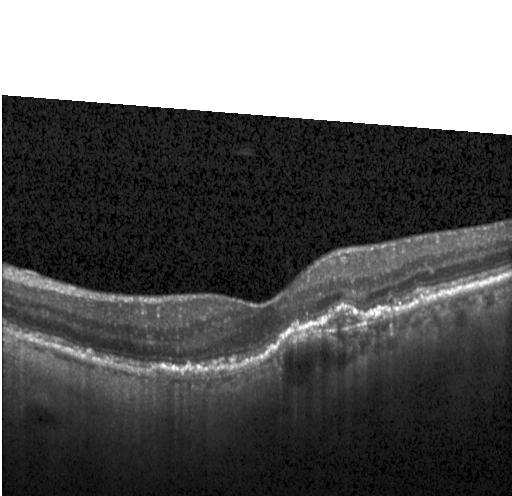 OCT line scan · spectral-domain OCT.
Dx: CNV.